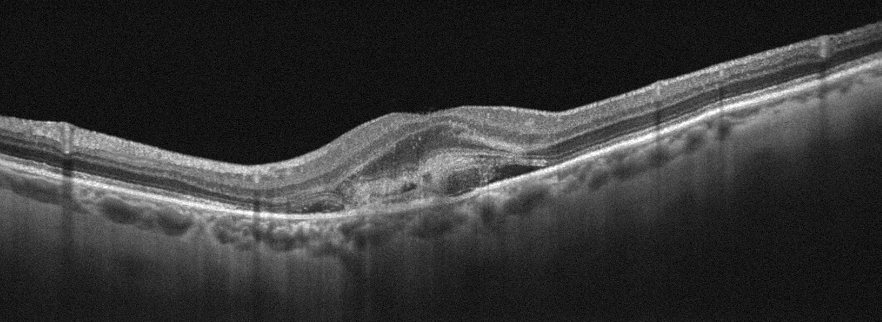 Left eye, retinal OCT cross-section
Impression: age-related macular degeneration (AMD).